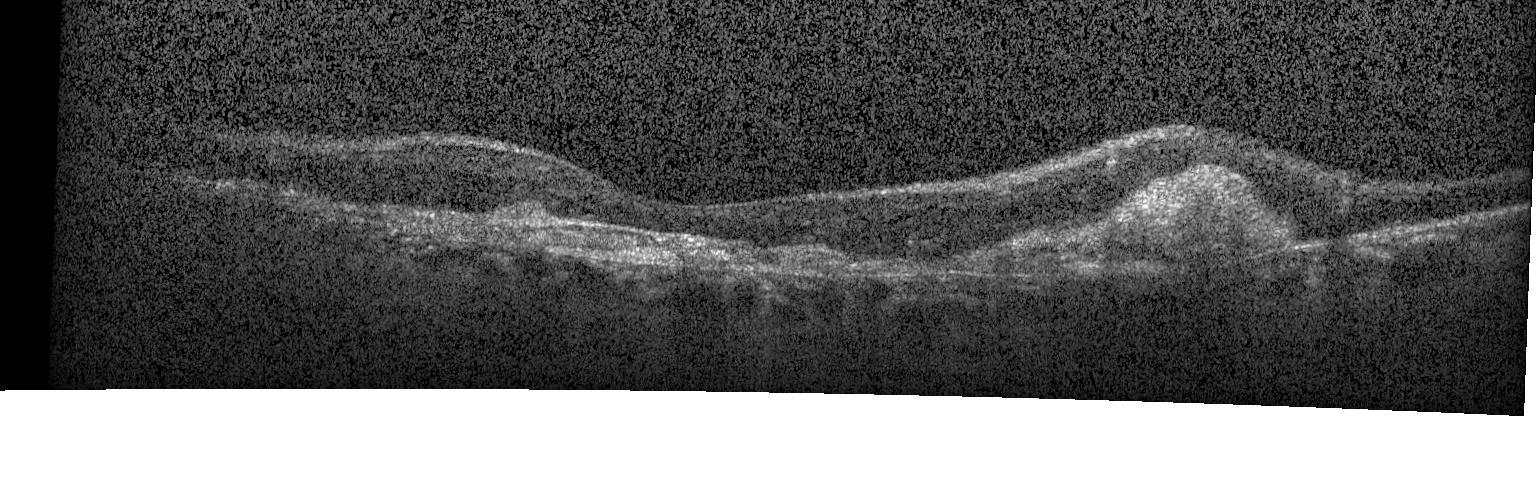

OCT finding: a choroidal neovascular membrane.